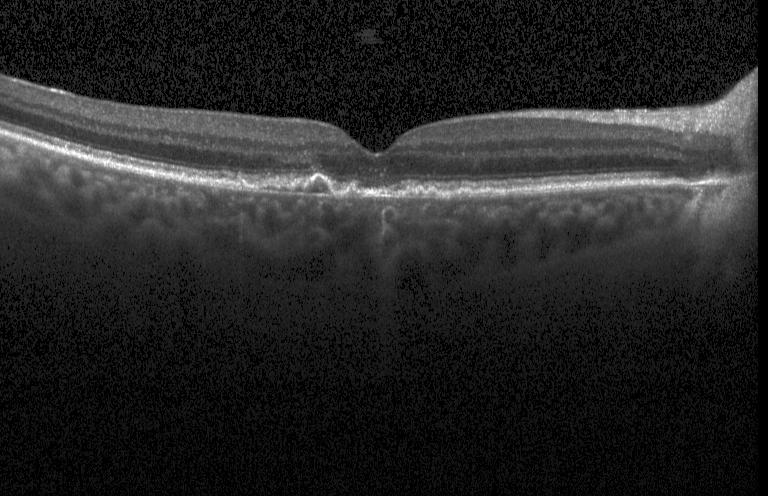 Spectral-domain optical coherence tomography, retinal OCT cross-section, Heidelberg Spectralis, centered on the fovea.
Assessment: choroidal neovascularization.